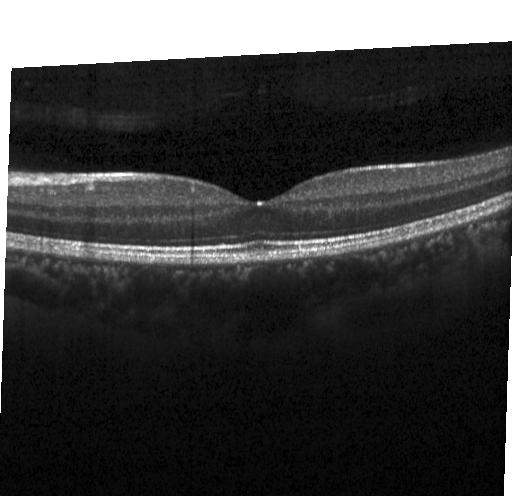
Optical coherence tomography scan; spectral-domain OCT.
Dx: no choroidal neovascularization, no diabetic macular edema, and no drusen.